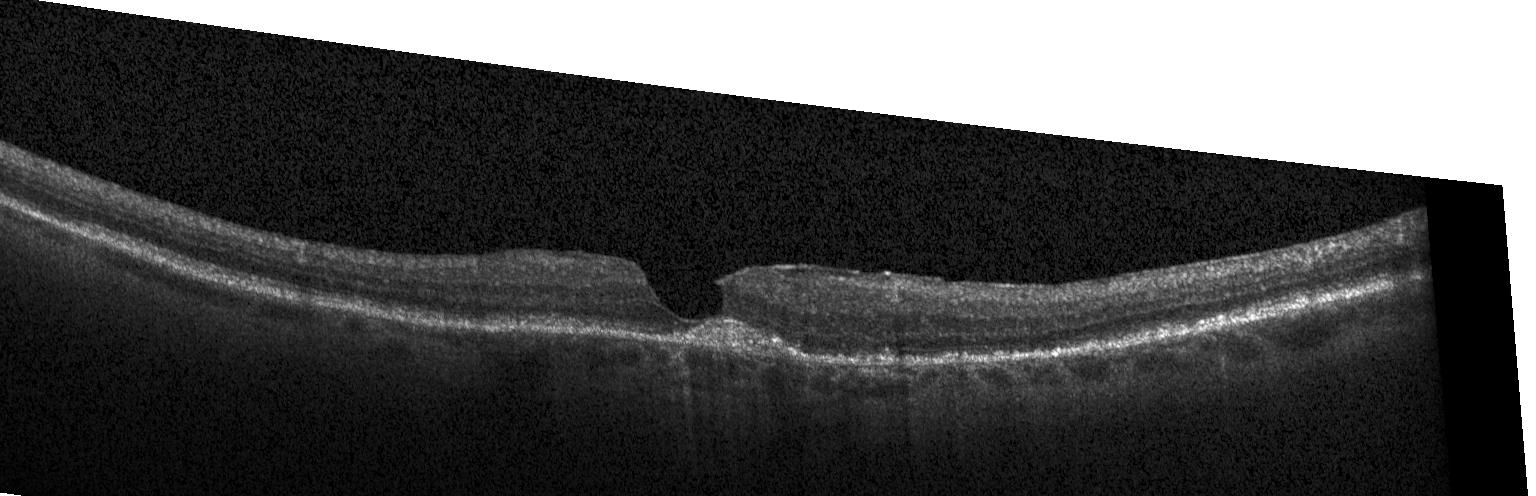 Retinal OCT cross-section showing a choroidal neovascular membrane.